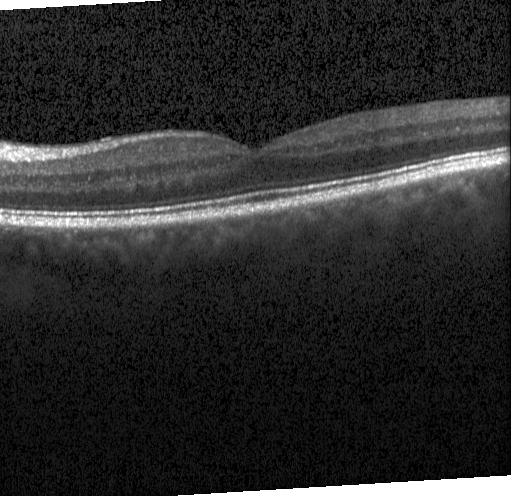

OCT line scan — Impression: neither choroidal neovascularization, diabetic macular edema, nor drusen.